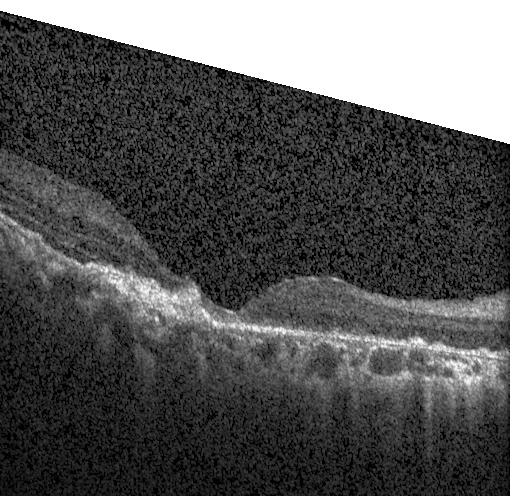
Heidelberg Spectralis OCT system. Spectral-domain optical coherence tomography. Horizontal scan through the fovea. Retinal OCT B-scan. The scan shows a choroidal neovascular membrane.